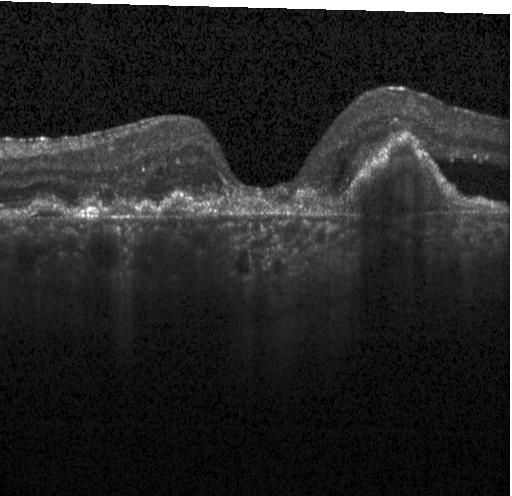

Spectral-domain optical coherence tomography, optical coherence tomography scan, acquired on a Heidelberg Spectralis. Impression: a choroidal neovascular membrane.